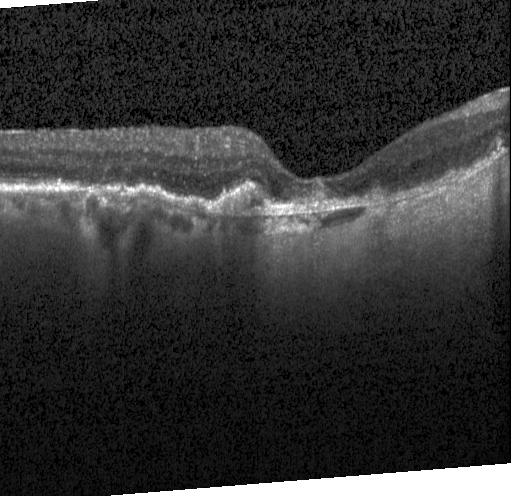
Spectral-domain OCT; retinal OCT cross-section. This B-scan demonstrates CNV.